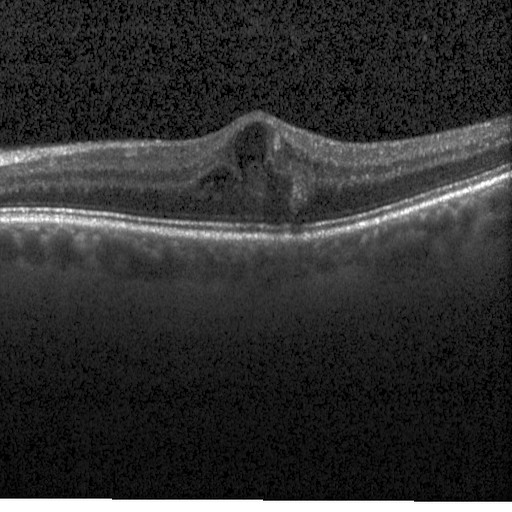 Spectral-domain OCT B-scan: diabetic macular edema (DME).